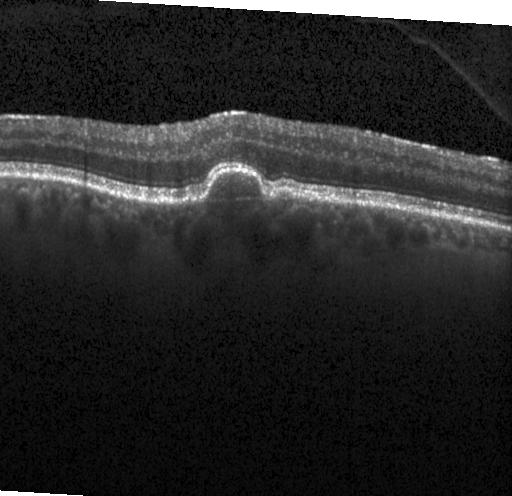
Optical coherence tomography scan. Macular scan. SD-OCT. Impression: a choroidal neovascular membrane.